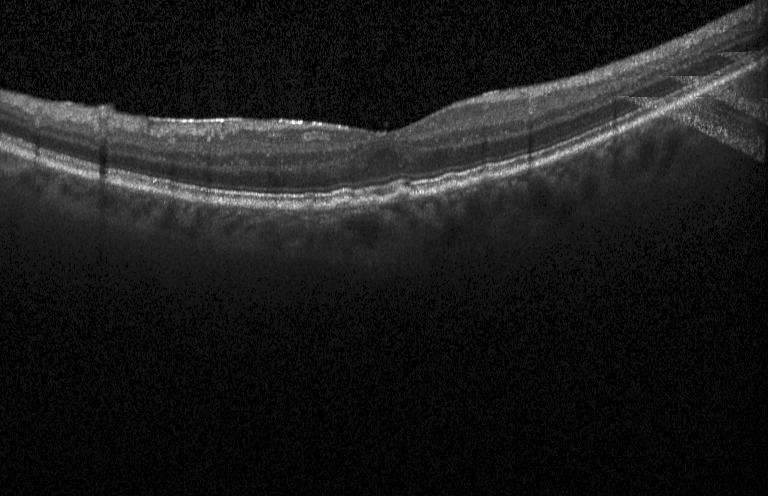
The scan shows multiple drusen.